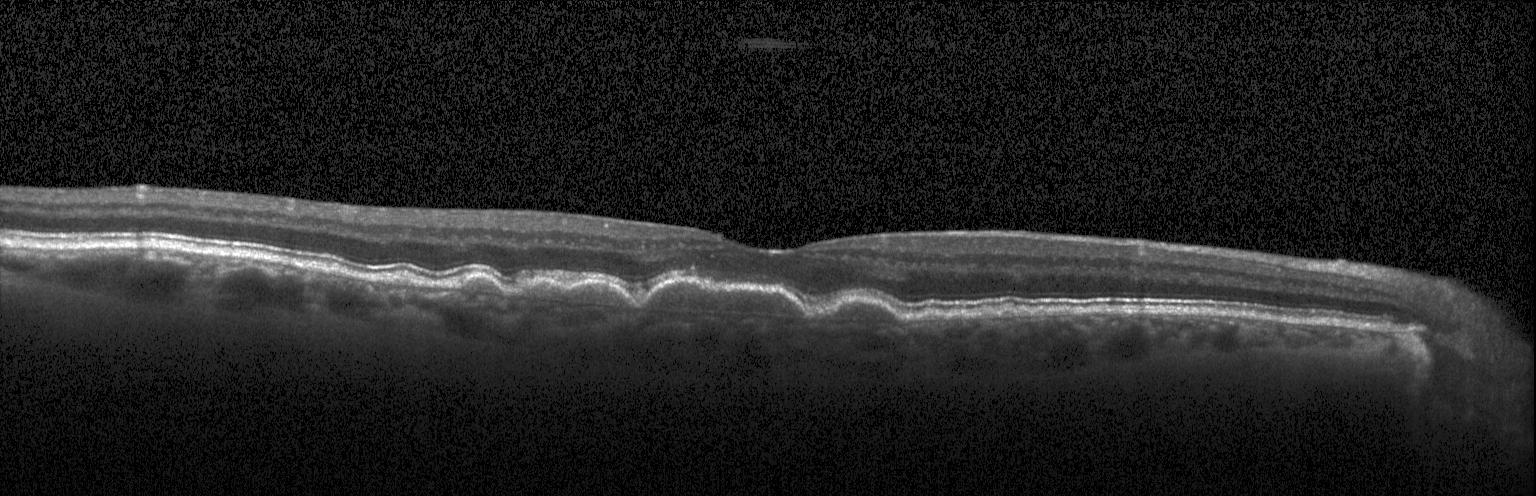
Macular OCT demonstrating multiple drusen.